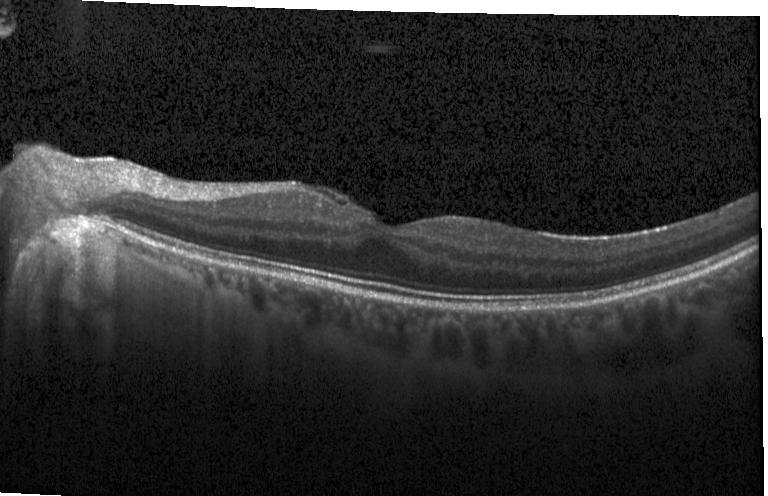
Retinal OCT cross-section · acquired on a Heidelberg Spectralis · fovea-centered
Macular OCT: no evidence of choroidal neovascularization, diabetic macular edema, or drusen.